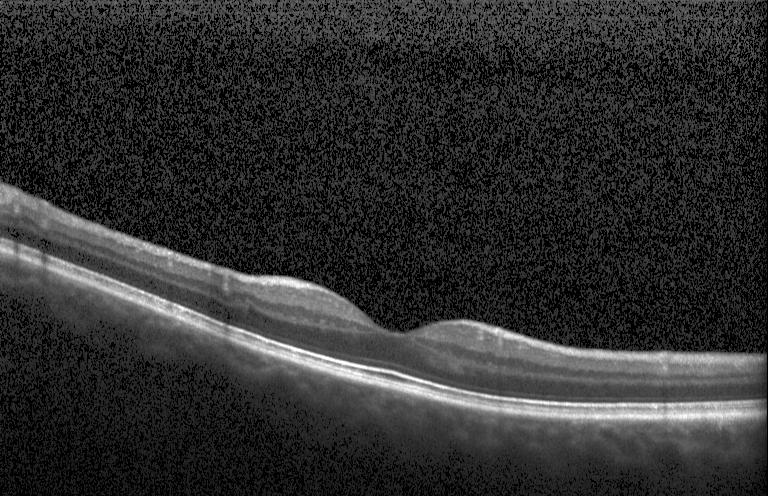
Retinal OCT cross-section
Finding: neither CNV, DME, nor drusen.